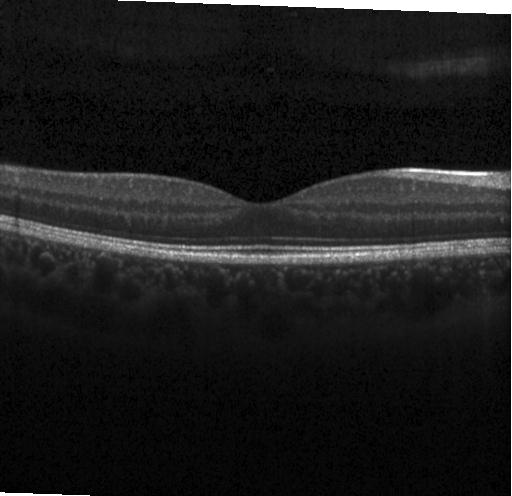

OCT B-scan, macular scan. Finding: no choroidal neovascularization, diabetic macular edema, or drusen.